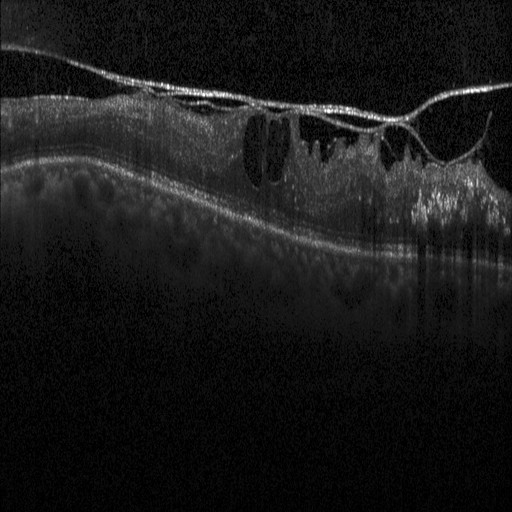

Retinal OCT cross-section showing diabetic macular edema (DME).